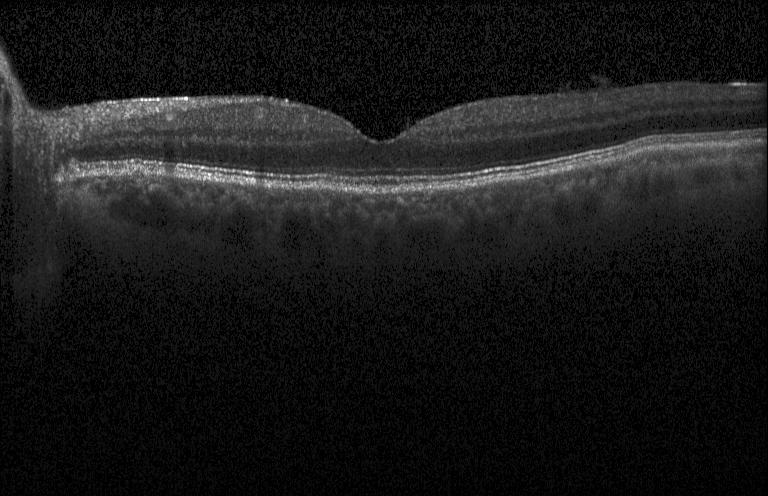 OCT line scan, macular scan, instrument: Heidelberg Spectralis. Impression: no choroidal neovascularization, no diabetic macular edema, and no drusen.